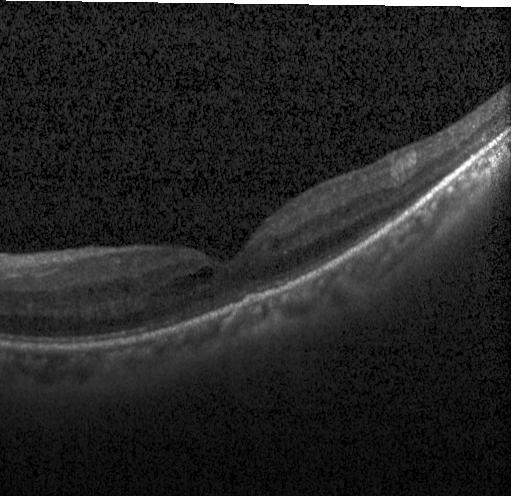

Assessment: DME.